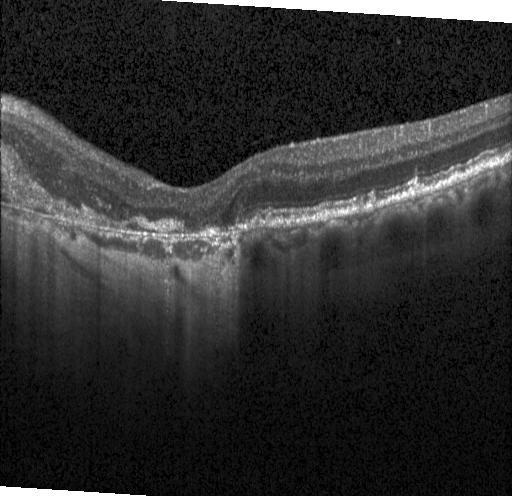 OCT line scan — Diagnosis: choroidal neovascularization.